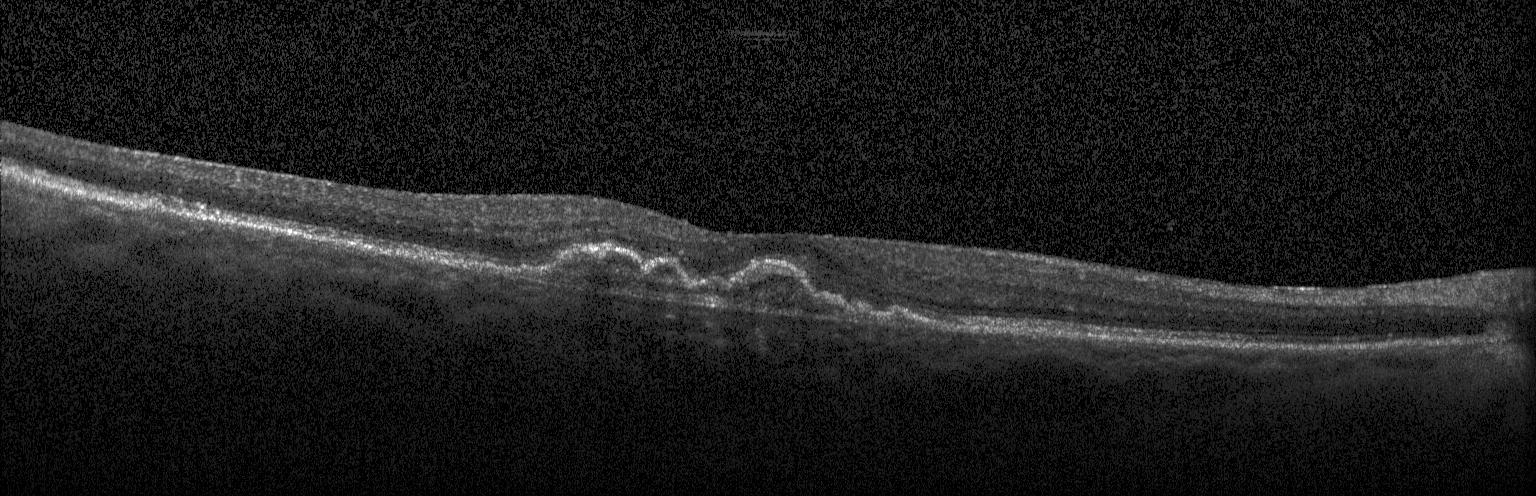
OCT line scan — Diagnosis: choroidal neovascularization.